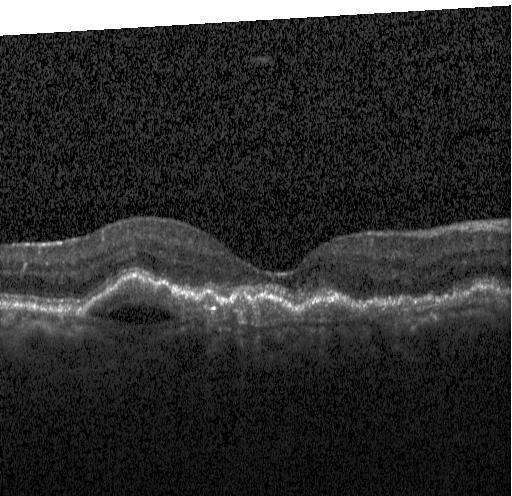 Retinal OCT B-scan · instrument: Heidelberg Spectralis · spectral-domain optical coherence tomography. Diagnosis: CNV.